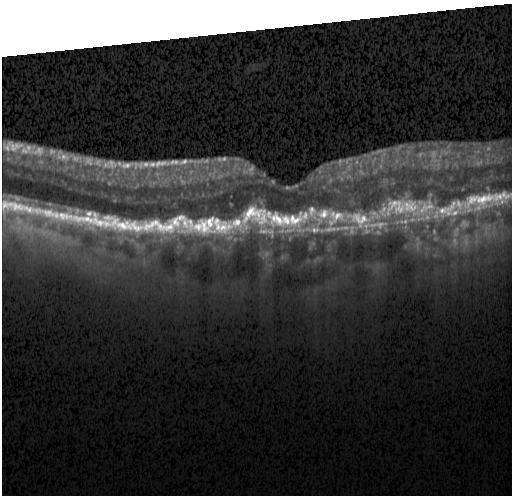 Finding: a choroidal neovascular membrane.